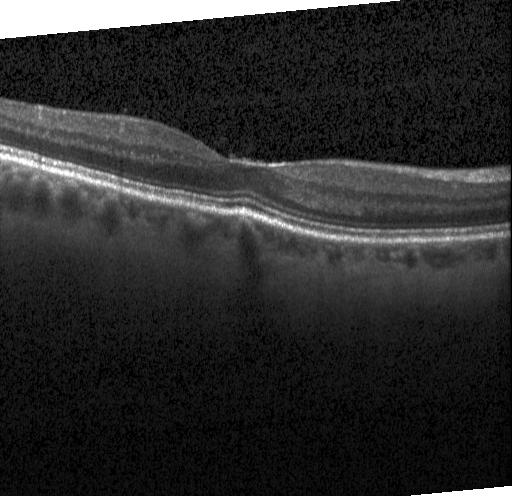
Fovea-centered; OCT B-scan
Diagnosis: no choroidal neovascularization, diabetic macular edema, or drusen.